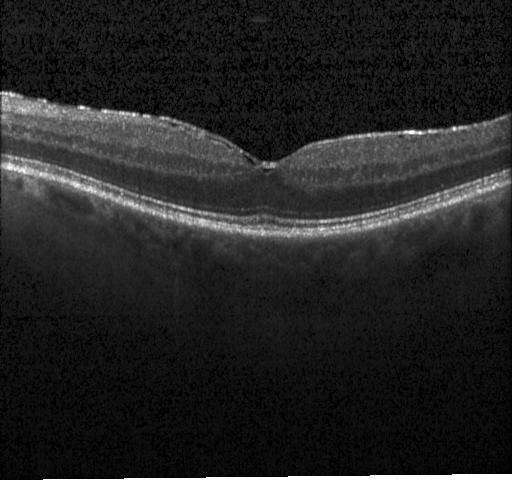
Retinal OCT cross-section · Heidelberg Spectralis · horizontal scan through the fovea. This B-scan demonstrates no evidence of choroidal neovascularization, diabetic macular edema, or drusen.